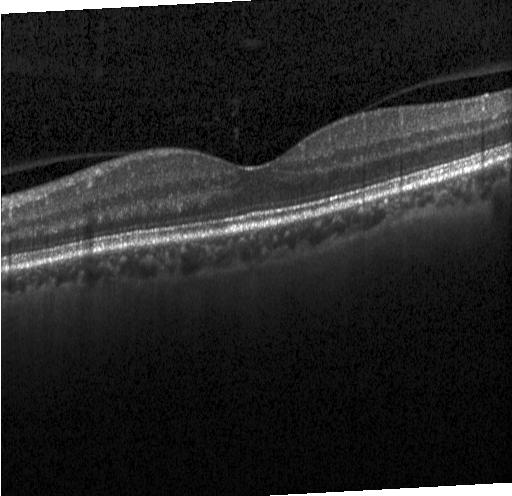 Heidelberg Spectralis OCT system, retinal OCT cross-section — Dx: no choroidal neovascularization, diabetic macular edema, or drusen.